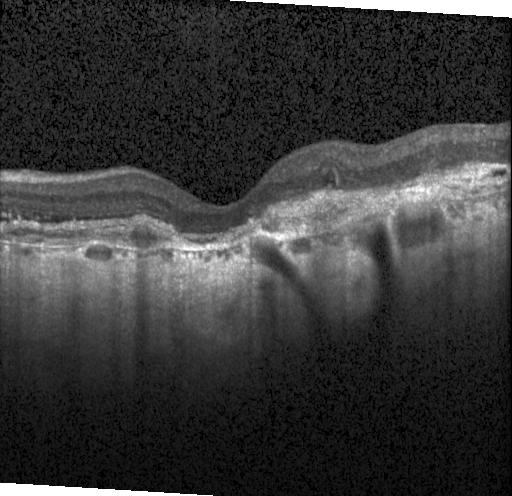

Spectral-domain OCT B-scan: a choroidal neovascular membrane.